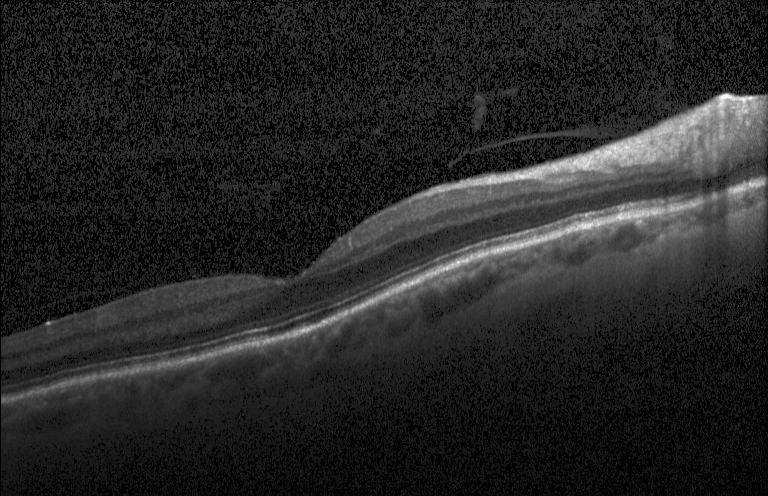 Centered on the fovea; optical coherence tomography scan; SD-OCT; Heidelberg Spectralis OCT system
No choroidal neovascularization, diabetic macular edema, or drusen.